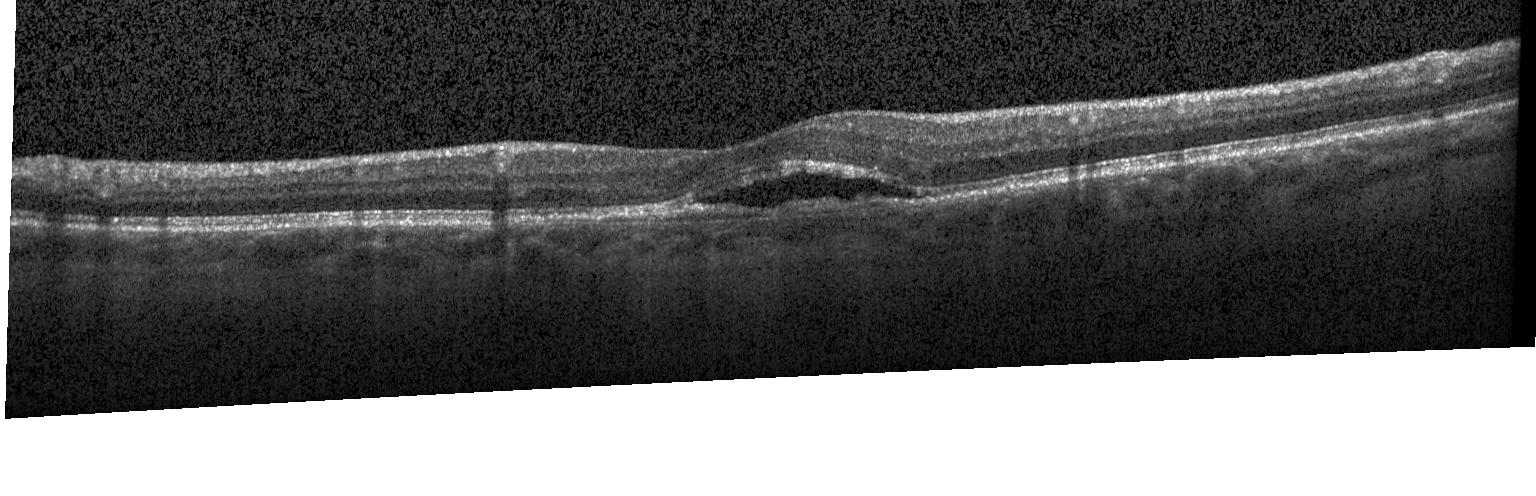 Acquired on a Heidelberg Spectralis; spectral-domain optical coherence tomography; optical coherence tomography scan.
Choroidal neovascularization (CNV).